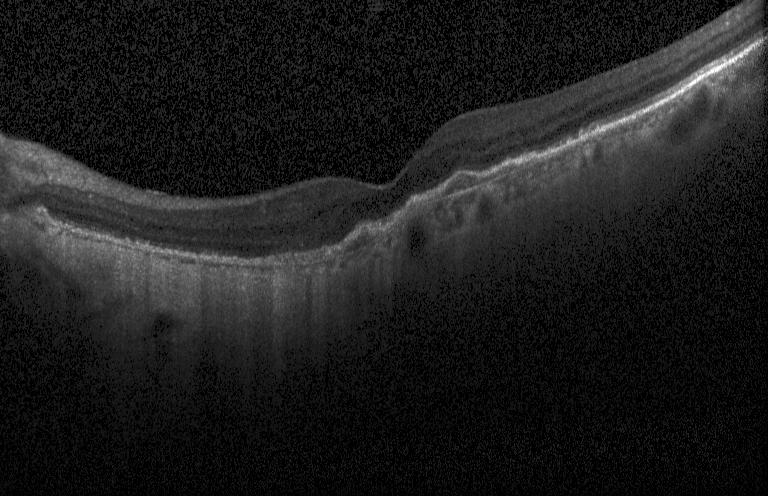

Instrument: Heidelberg Spectralis. OCT line scan
Finding: a choroidal neovascular membrane.